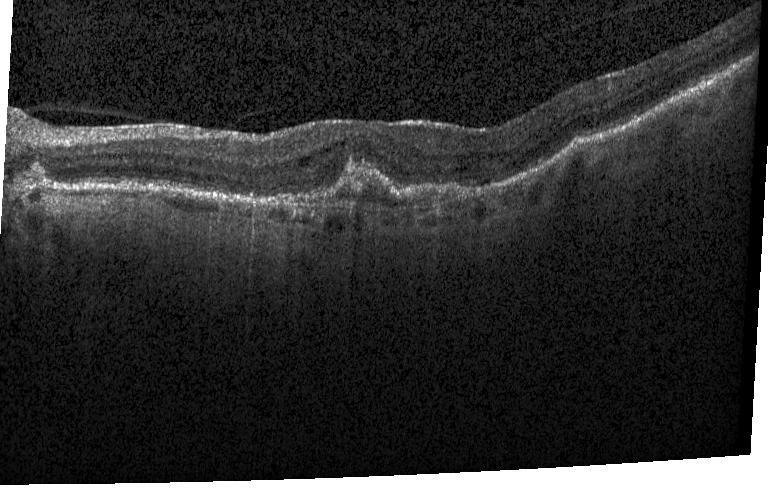

Optical coherence tomography B-scan — Finding: a choroidal neovascular membrane.